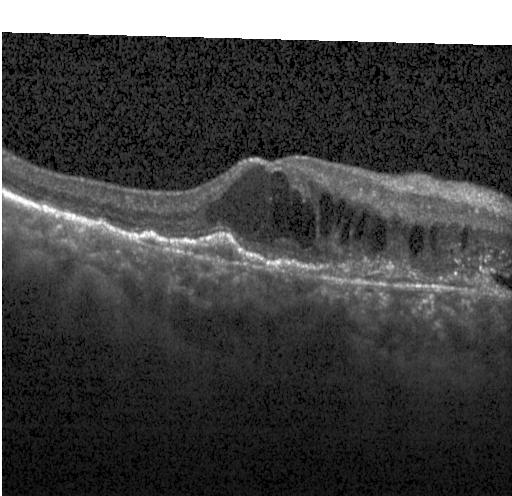
OCT scan showing CNV.